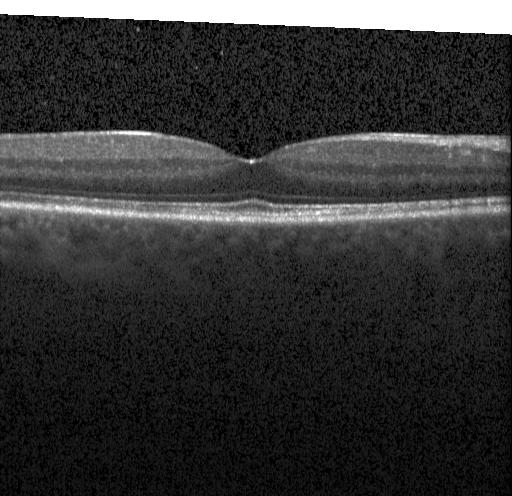 Finding: no evidence of choroidal neovascularization, diabetic macular edema, or drusen.